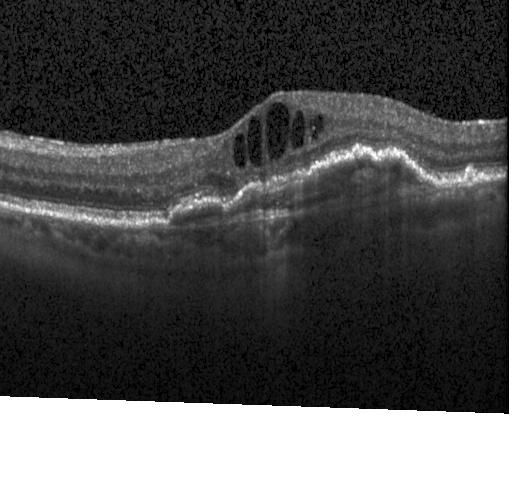

Retinal OCT B-scan; fovea-centered
Impression: a choroidal neovascular membrane.